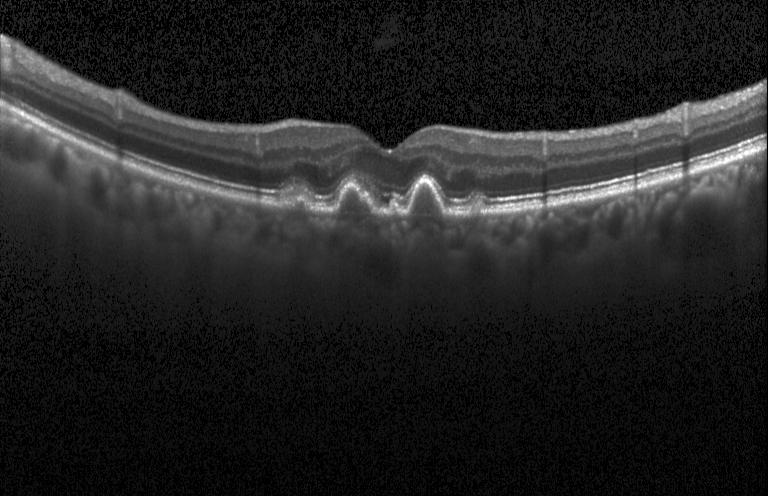
Spectral-domain OCT. Optical coherence tomography scan
Drusen.